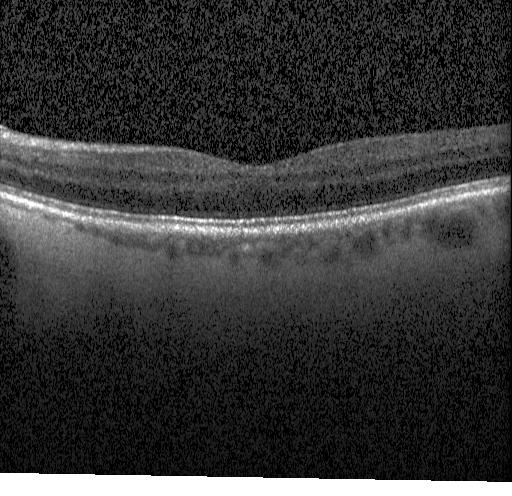
OCT line scan · fovea-centered.
The scan shows no choroidal neovascularization, diabetic macular edema, or drusen.